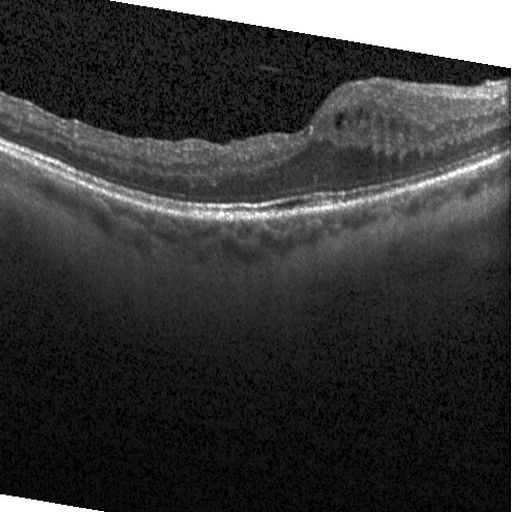
Diagnosis: diabetic macular edema.